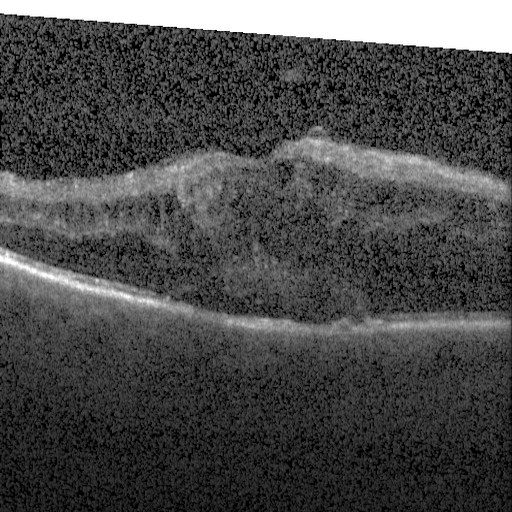

Macular OCT demonstrating DME.